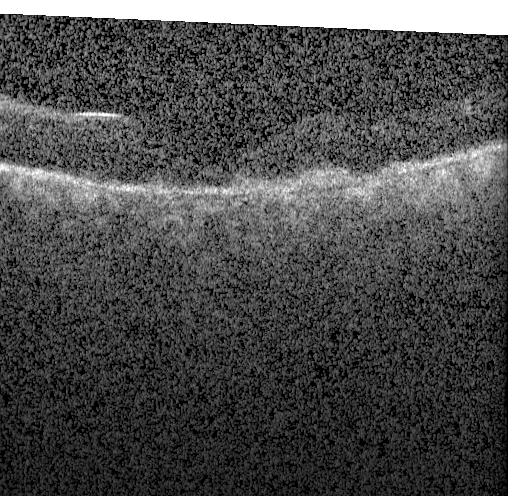 Retinal OCT B-scan. Heidelberg Spectralis.
Impression: a choroidal neovascular membrane.